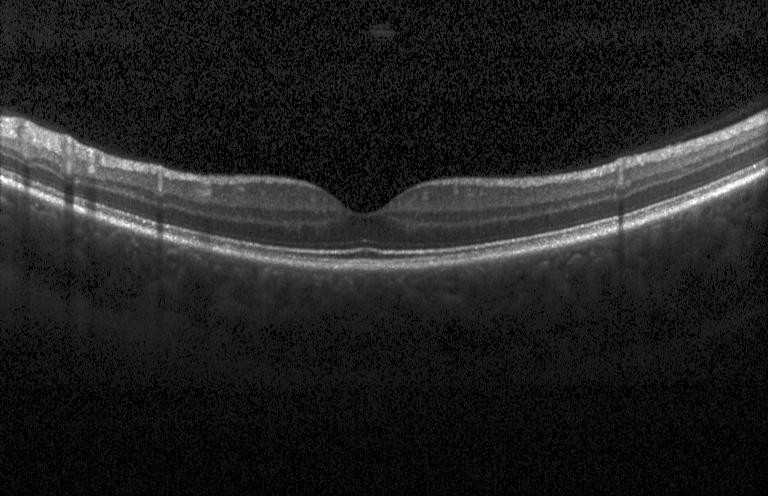 Through the macula · OCT B-scan · SD-OCT — This B-scan demonstrates no choroidal neovascularization, no diabetic macular edema, and no drusen.